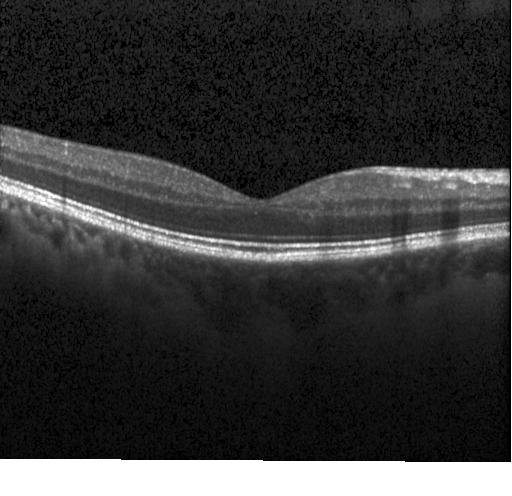 Finding: no evidence of CNV, DME, or drusen.